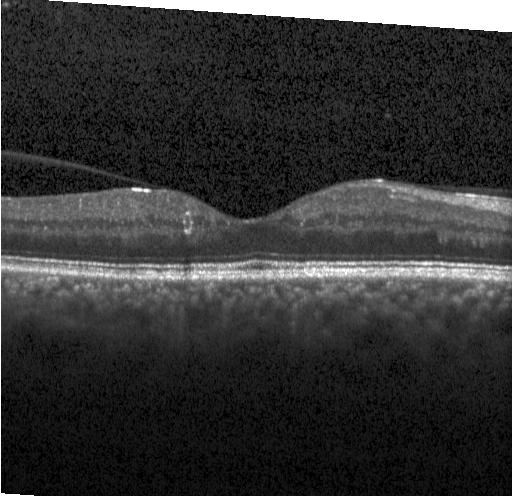 Finding: neither choroidal neovascularization, diabetic macular edema, nor drusen.